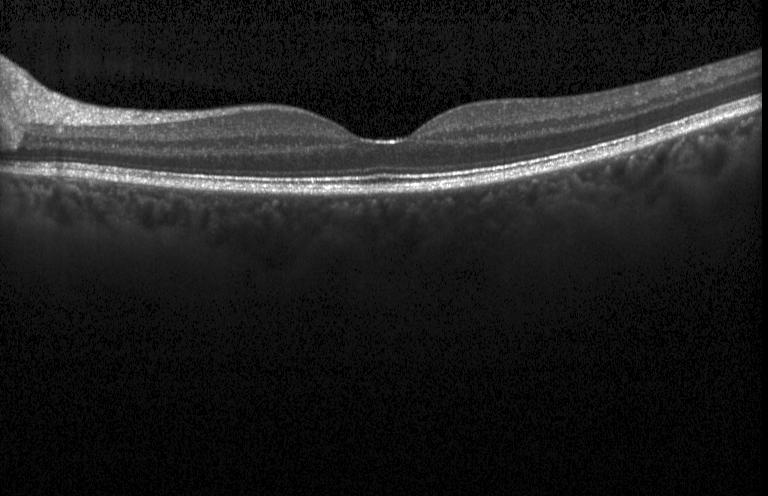
OCT B-scan; centered on the fovea; instrument: Heidelberg Spectralis.
Diagnosis: no evidence of choroidal neovascularization, diabetic macular edema, or drusen.